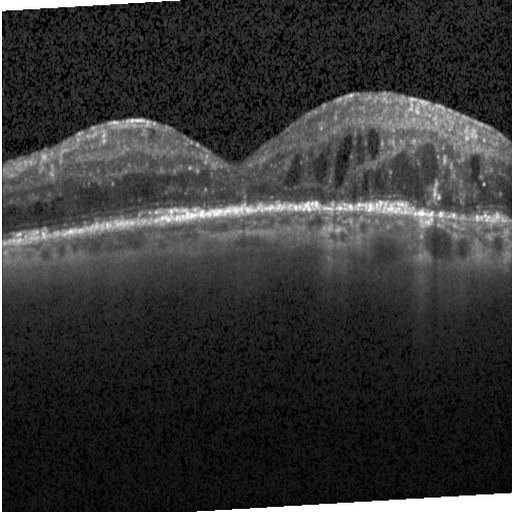

OCT line scan · spectral-domain optical coherence tomography. Diagnosis: diabetic macular edema.